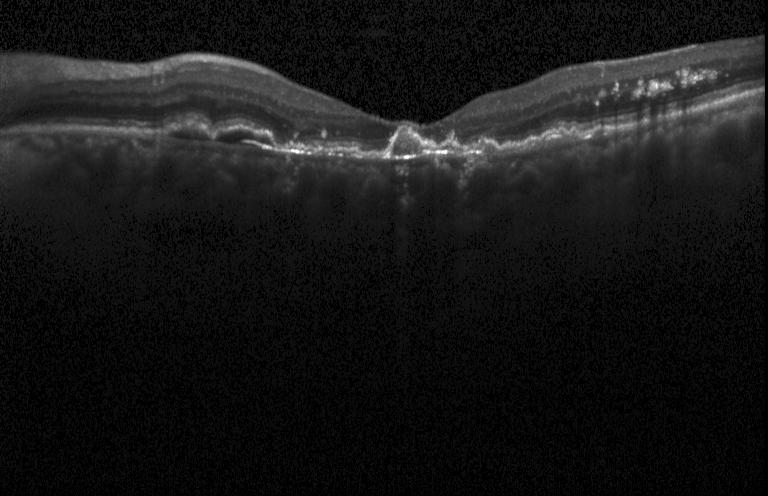

OCT finding: a choroidal neovascular membrane.